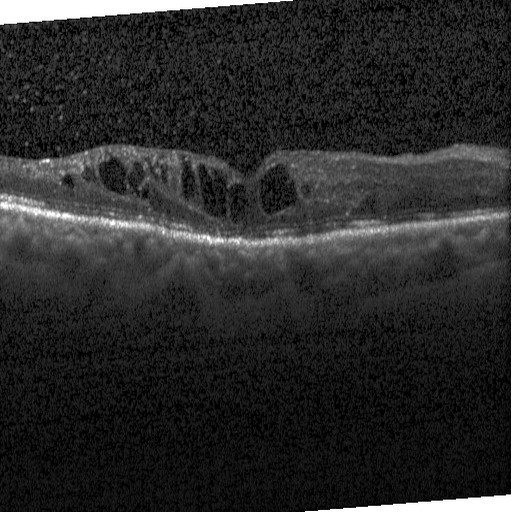

Horizontal scan through the fovea, optical coherence tomography scan — Assessment: diabetic macular edema.